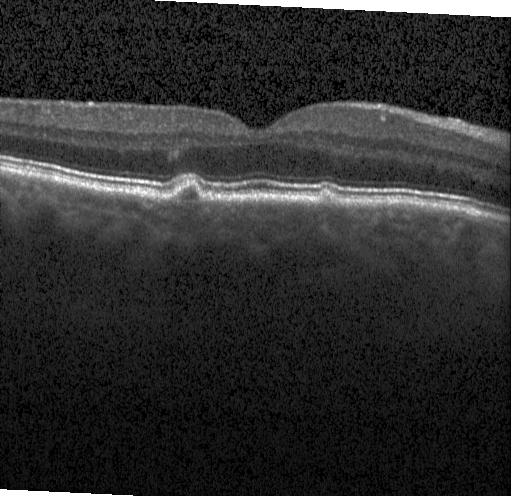
Optical coherence tomography B-scan. Spectral-domain optical coherence tomography. Heidelberg Spectralis. Finding: sub-RPE drusenoid deposits.